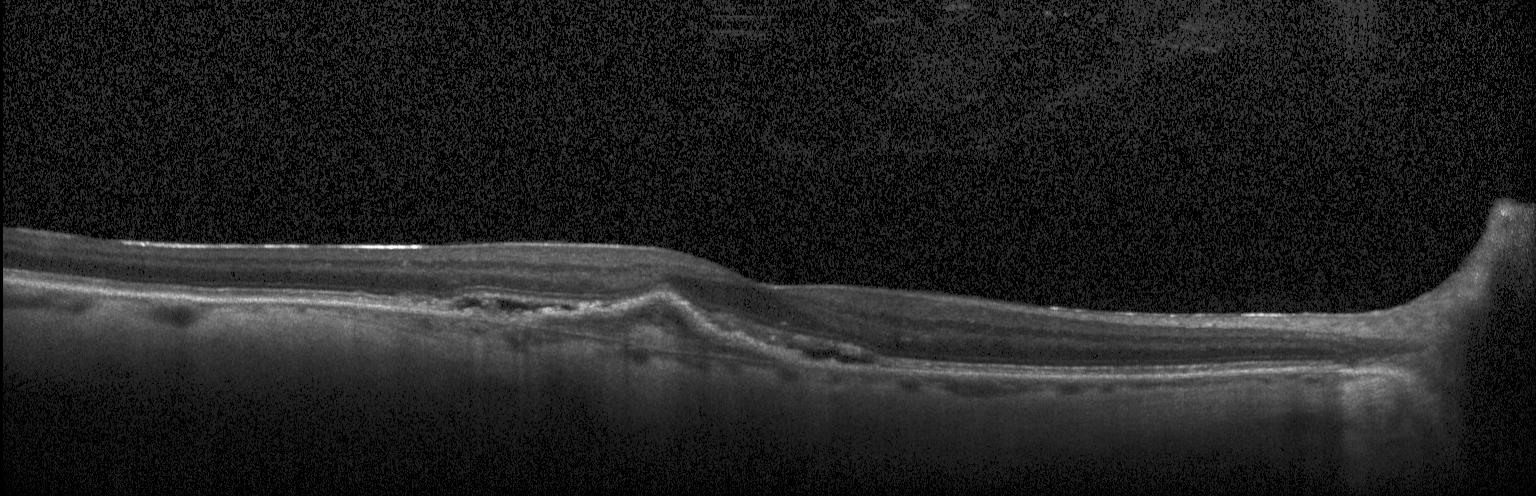

This B-scan demonstrates a choroidal neovascular membrane.